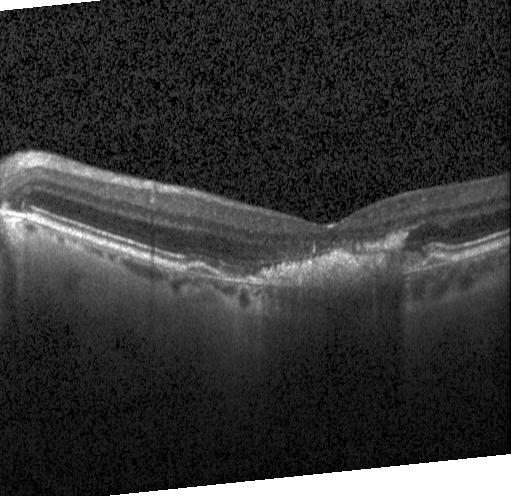 Fovea-centered. Acquired on a Heidelberg Spectralis. Optical coherence tomography B-scan
A choroidal neovascular membrane.